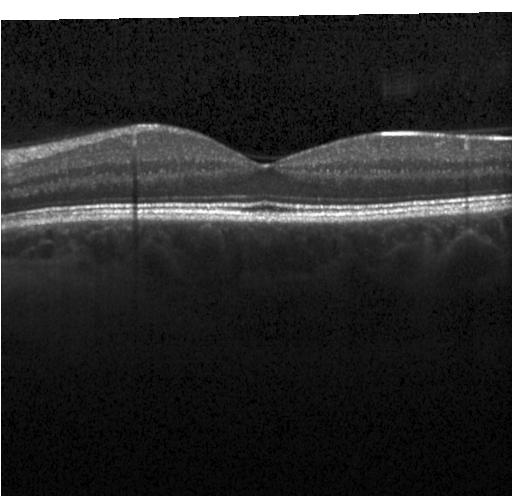

OCT B-scan showing no CNV, no DME, and no drusen.